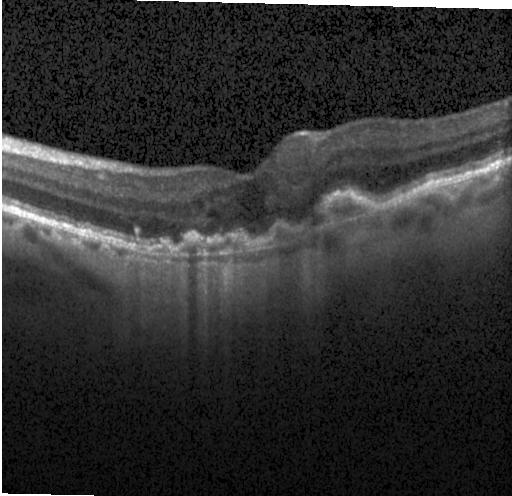
Spectral-domain OCT; retinal OCT B-scan; centered on the fovea; acquired on a Heidelberg Spectralis. Diagnosis: choroidal neovascularization.